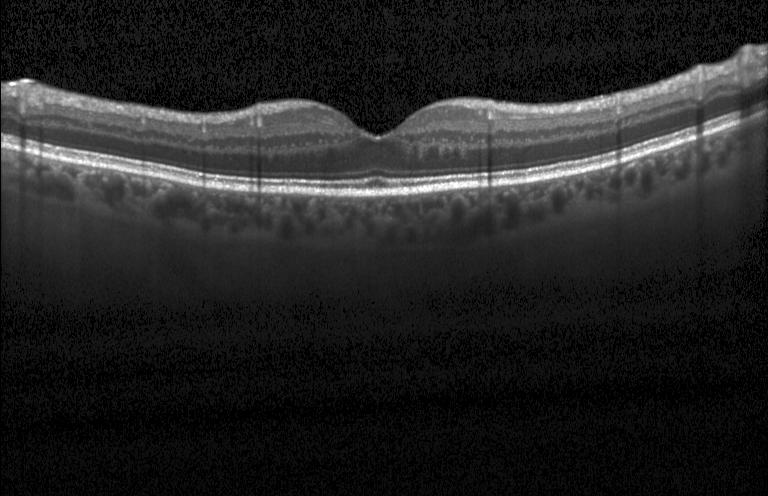
This B-scan demonstrates neither choroidal neovascularization, diabetic macular edema, nor drusen.